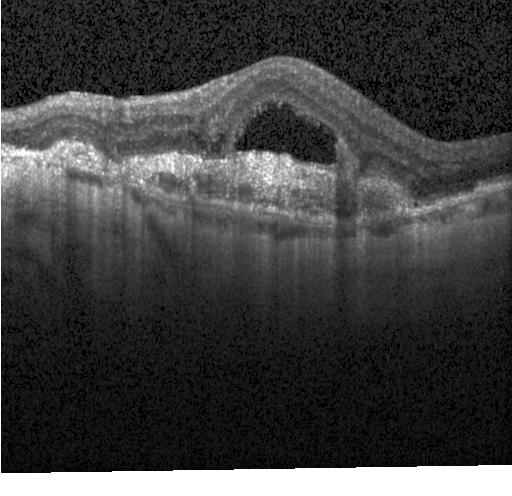 Retinal OCT cross-section; Heidelberg Spectralis; horizontal scan through the fovea; spectral-domain OCT. The scan shows choroidal neovascularization (CNV).